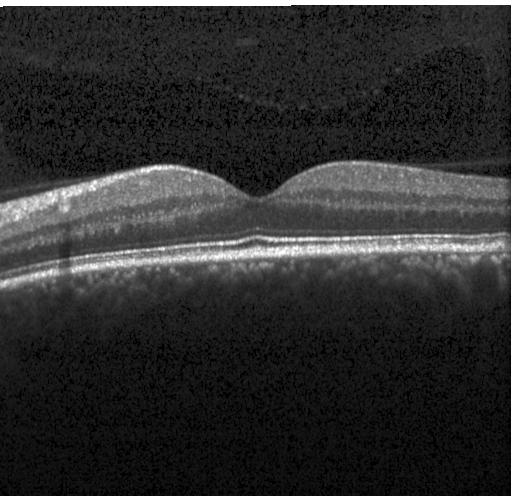

OCT B-scan; spectral-domain optical coherence tomography; fovea-centered; acquired on a Heidelberg Spectralis.
Finding: no CNV, DME, or drusen.